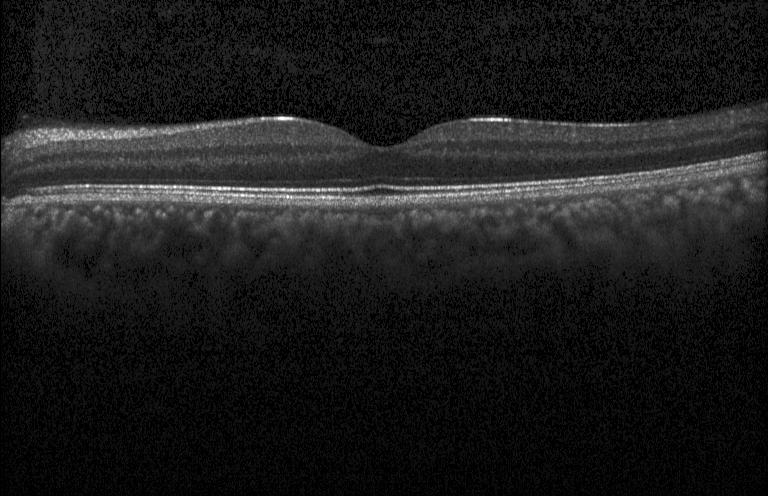
Spectral-domain OCT B-scan: neither choroidal neovascularization, diabetic macular edema, nor drusen.